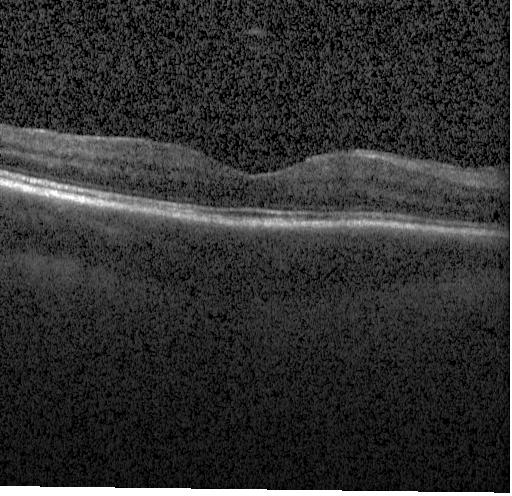
Spectral-domain OCT B-scan: no evidence of choroidal neovascularization, diabetic macular edema, or drusen.